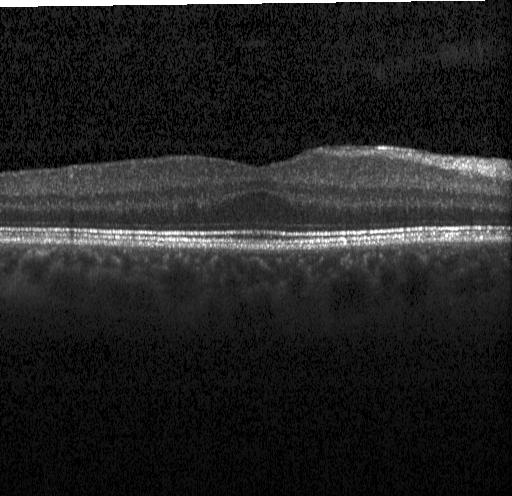

Acquired on a Heidelberg Spectralis, SD-OCT, optical coherence tomography B-scan
The scan shows no evidence of choroidal neovascularization, diabetic macular edema, or drusen.